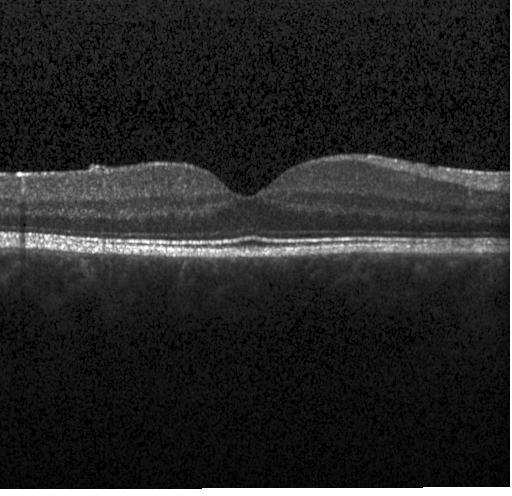

OCT line scan — This B-scan demonstrates neither choroidal neovascularization, diabetic macular edema, nor drusen.